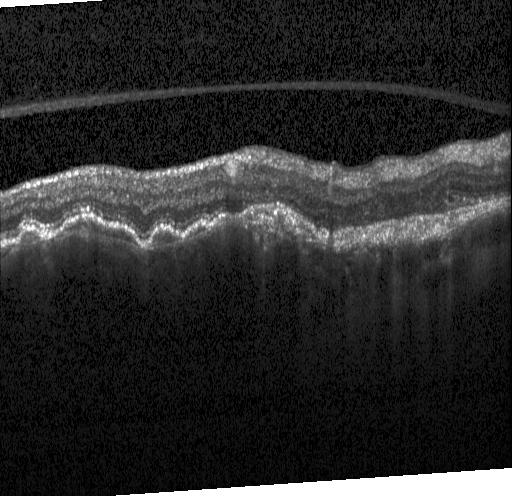

Spectral-domain optical coherence tomography. Horizontal scan through the fovea. Retinal OCT B-scan. Heidelberg Spectralis OCT system.
Diagnosis: a choroidal neovascular membrane.